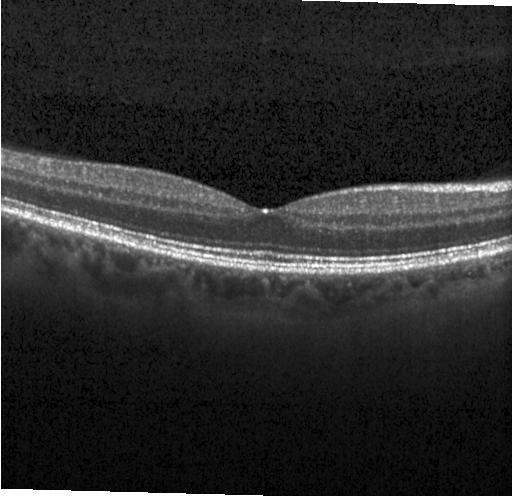

Diagnosis: no evidence of choroidal neovascularization, diabetic macular edema, or drusen.